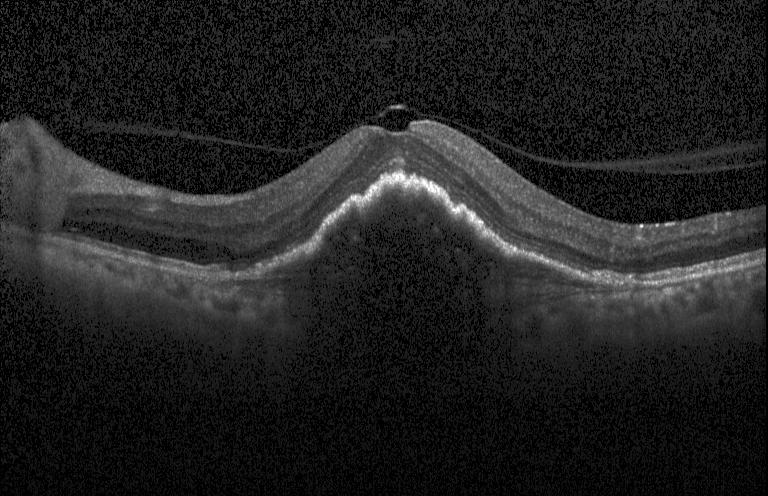
Impression: choroidal neovascularization (CNV).